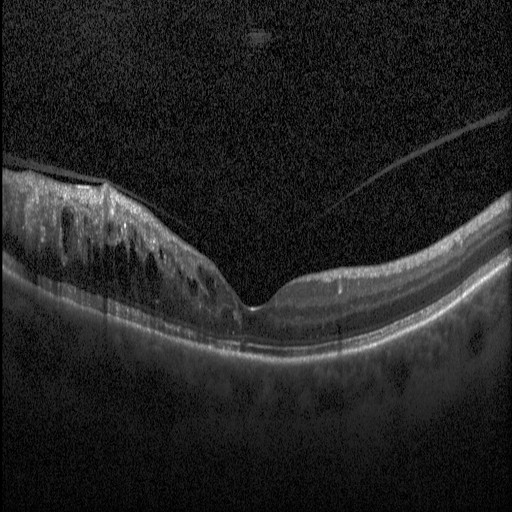

Through the macula. Optical coherence tomography B-scan. Heidelberg Spectralis — Dx: DME.